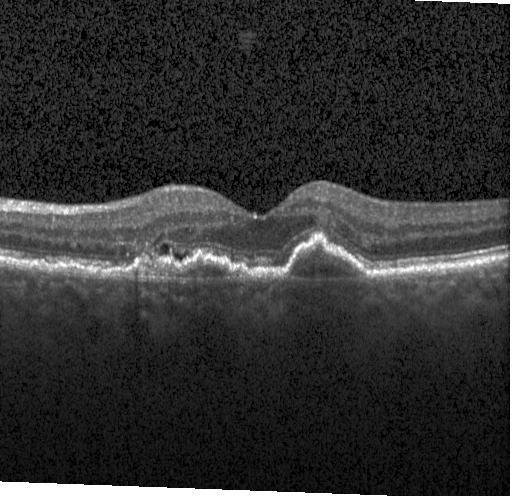 Impression: choroidal neovascularization (CNV).